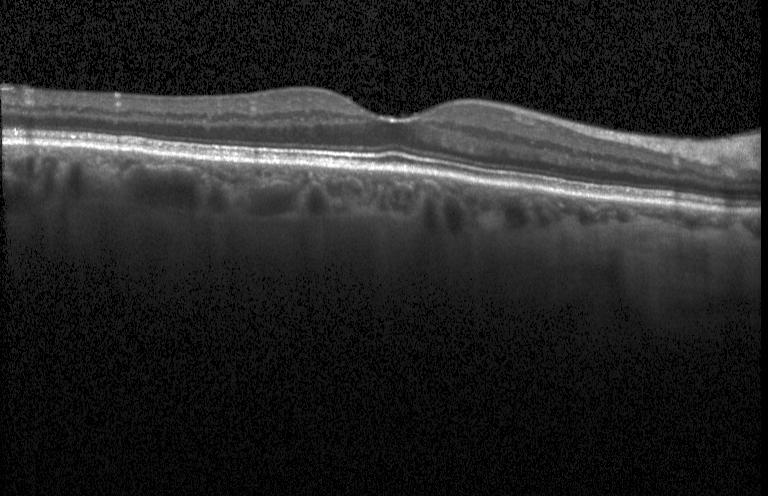

Retinal OCT cross-section showing no choroidal neovascularization, diabetic macular edema, or drusen.